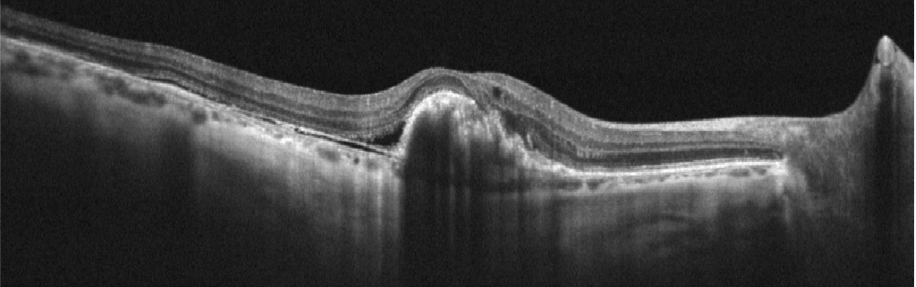

Optical coherence tomography scan. Age-related macular degeneration (AMD).